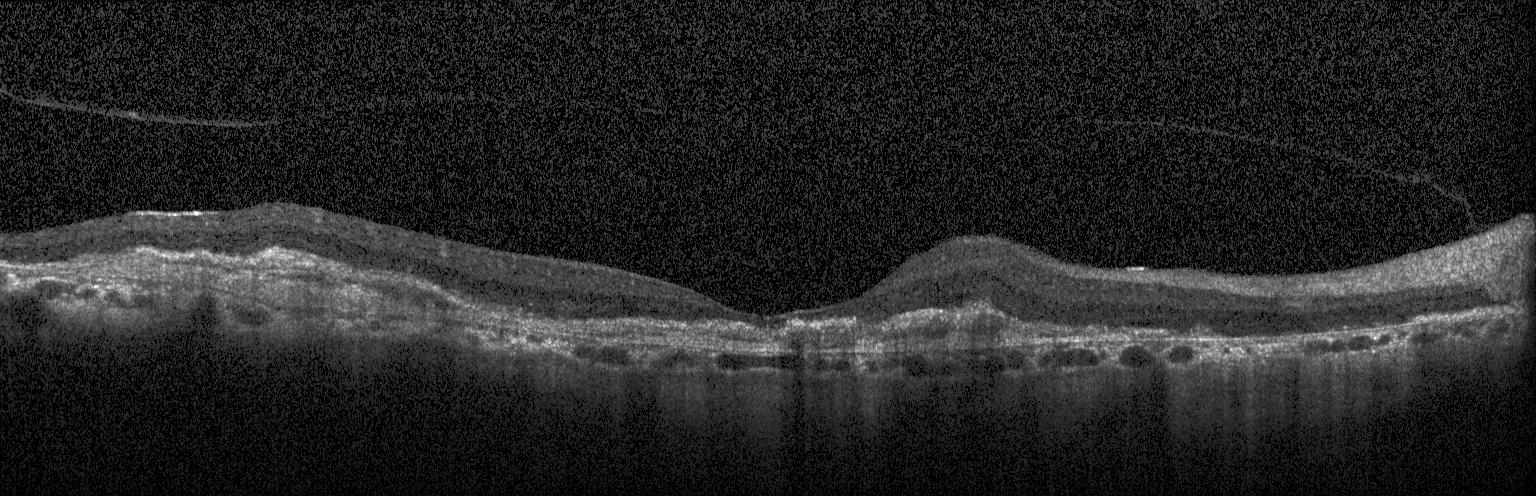

Optical coherence tomography scan · spectral-domain OCT · acquired on a Heidelberg Spectralis.
Dx: choroidal neovascularization (CNV).